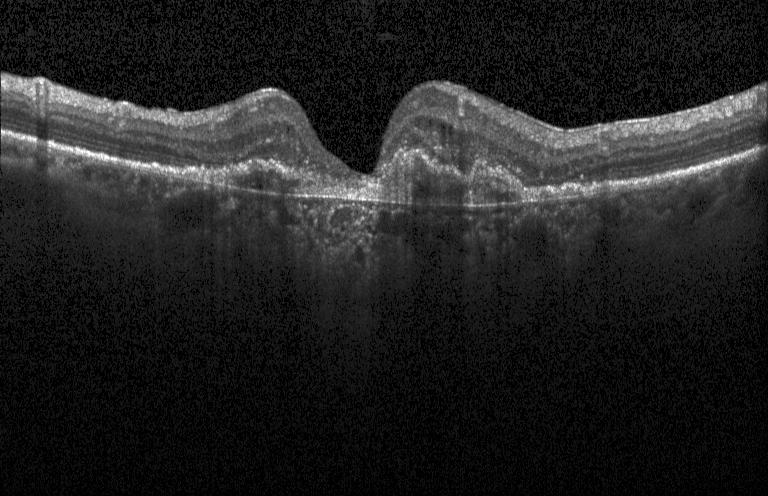

Acquired on a Heidelberg Spectralis · centered on the fovea · optical coherence tomography B-scan.
OCT finding: a choroidal neovascular membrane.